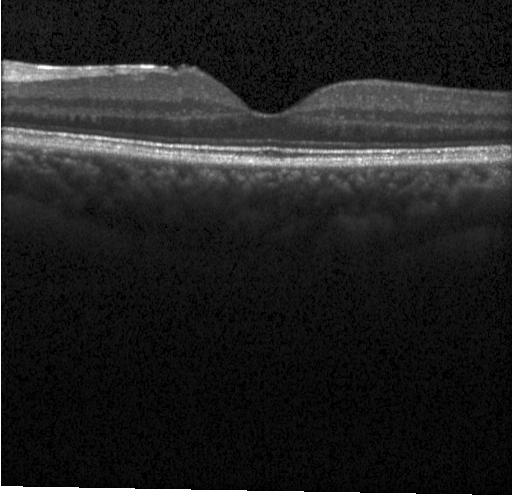
OCT scan showing no evidence of choroidal neovascularization, diabetic macular edema, or drusen.